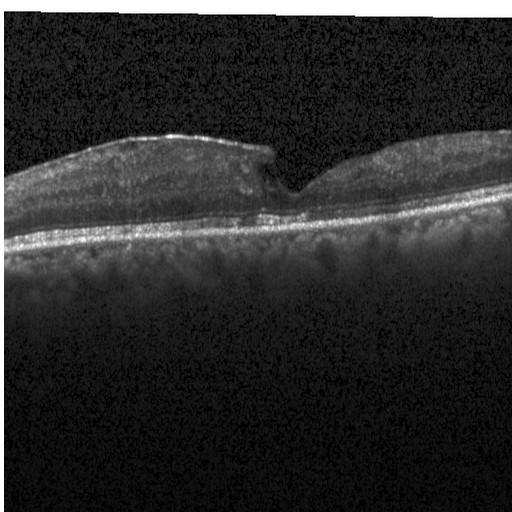

Horizontal scan through the fovea, retinal OCT cross-section, acquired on a Heidelberg Spectralis.
OCT finding: DME.